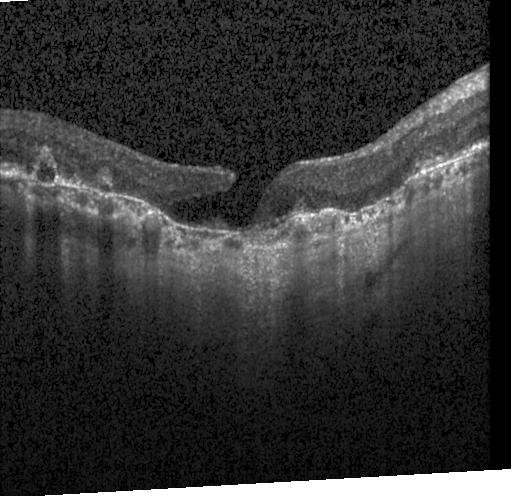 Heidelberg Spectralis OCT system · spectral-domain optical coherence tomography · retinal OCT cross-section
Macular OCT: CNV.